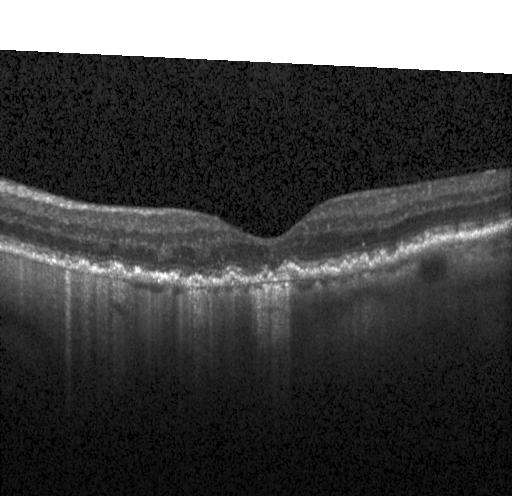
Impression: drusen.